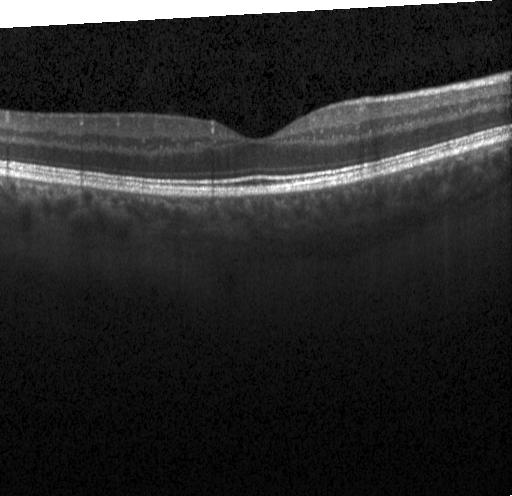

This B-scan demonstrates neither choroidal neovascularization, diabetic macular edema, nor drusen.